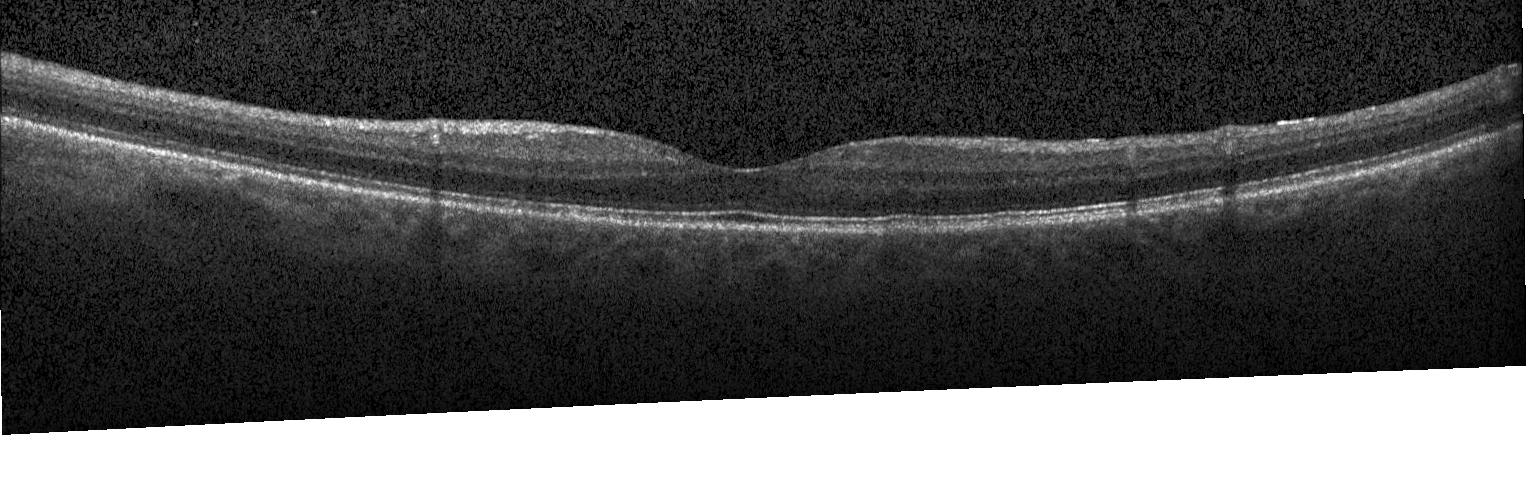
Assessment: neither choroidal neovascularization, diabetic macular edema, nor drusen.